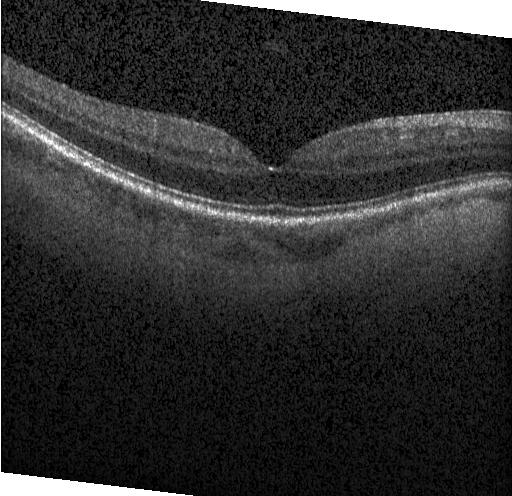

Acquired on a Heidelberg Spectralis. Macular scan. SD-OCT. OCT line scan — Assessment: no choroidal neovascularization, diabetic macular edema, or drusen.